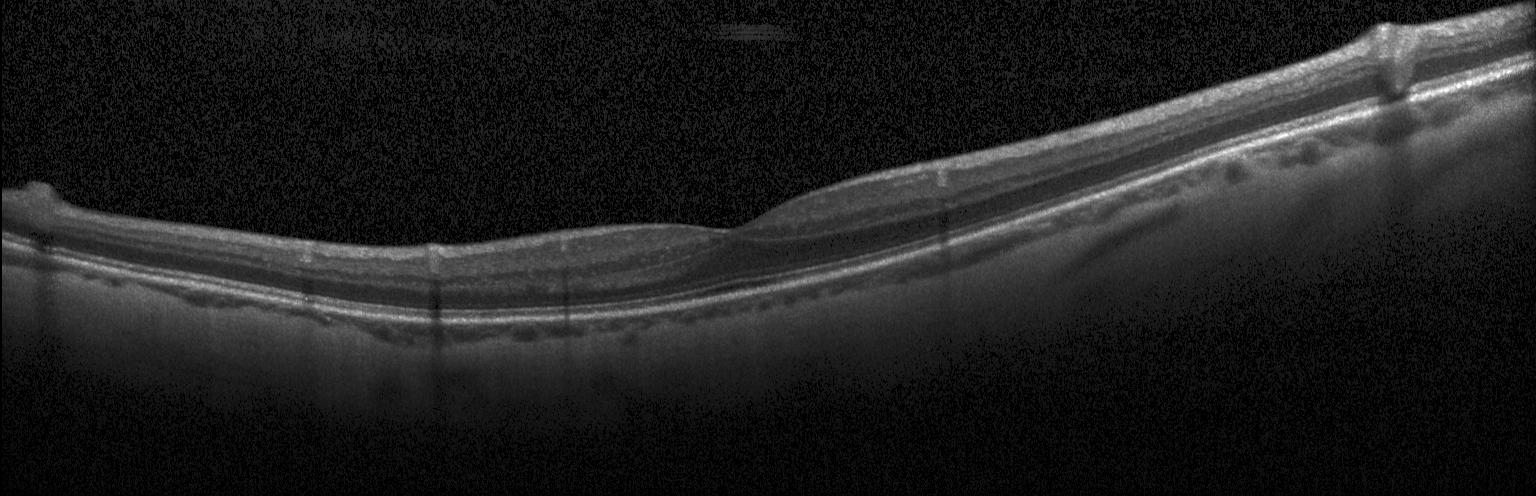
Dx: no choroidal neovascularization, no diabetic macular edema, and no drusen.